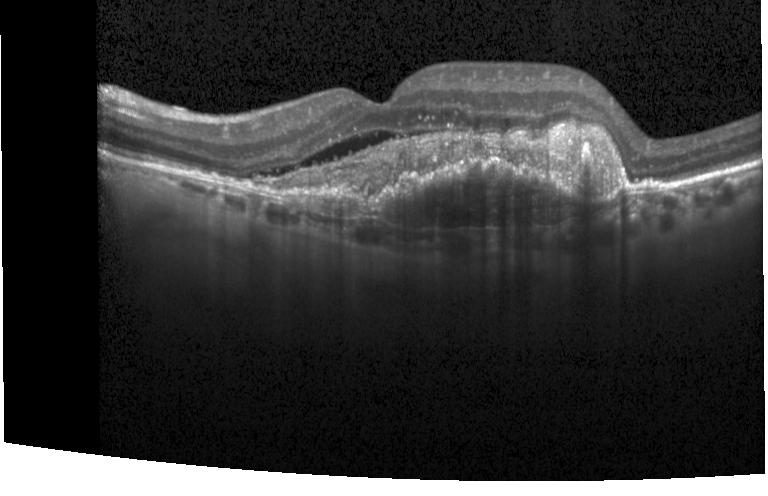
Retinal OCT cross-section.
Dx: choroidal neovascularization.